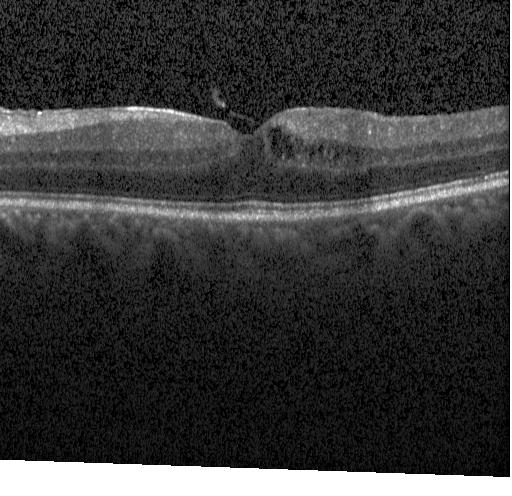 OCT B-scan. The scan shows diabetic macular edema (DME).